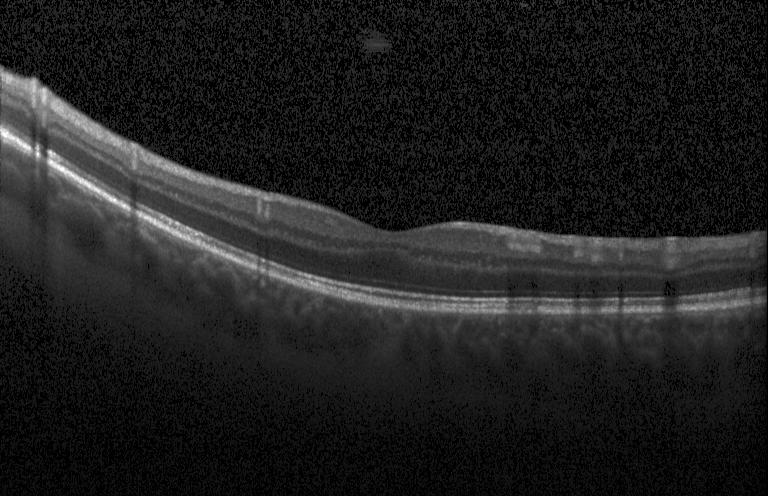
OCT scan showing no CNV, DME, or drusen.